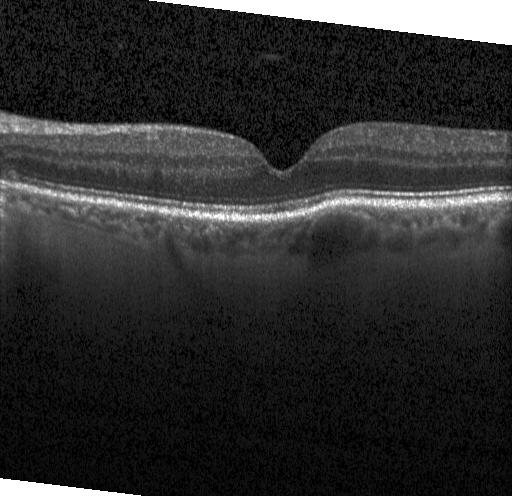 Optical coherence tomography scan. Spectral-domain optical coherence tomography. Heidelberg Spectralis. The scan shows no choroidal neovascularization, diabetic macular edema, or drusen.